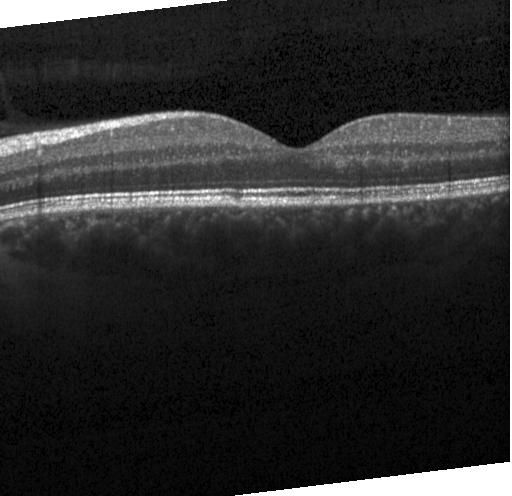 OCT B-scan showing neither choroidal neovascularization, diabetic macular edema, nor drusen.